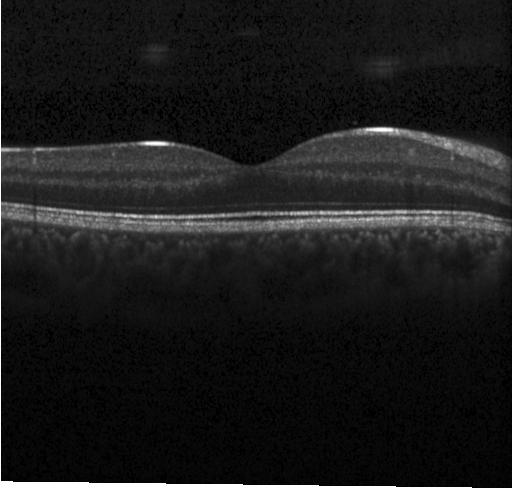

OCT finding: no evidence of choroidal neovascularization, diabetic macular edema, or drusen.